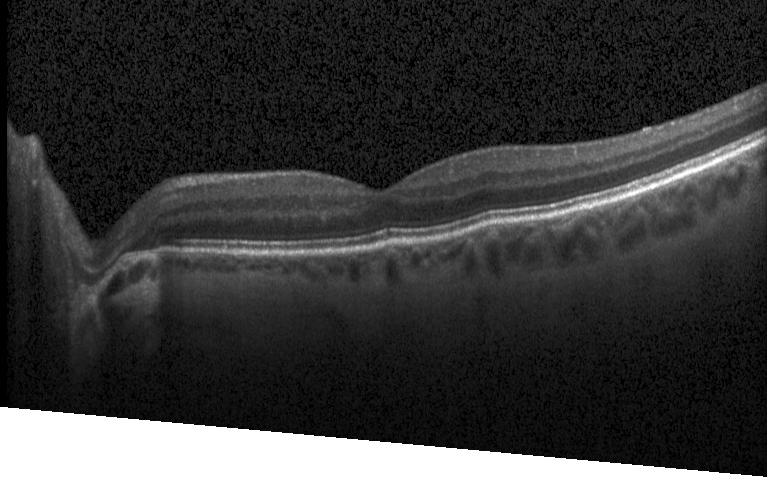 Finding: no CNV, no DME, and no drusen.